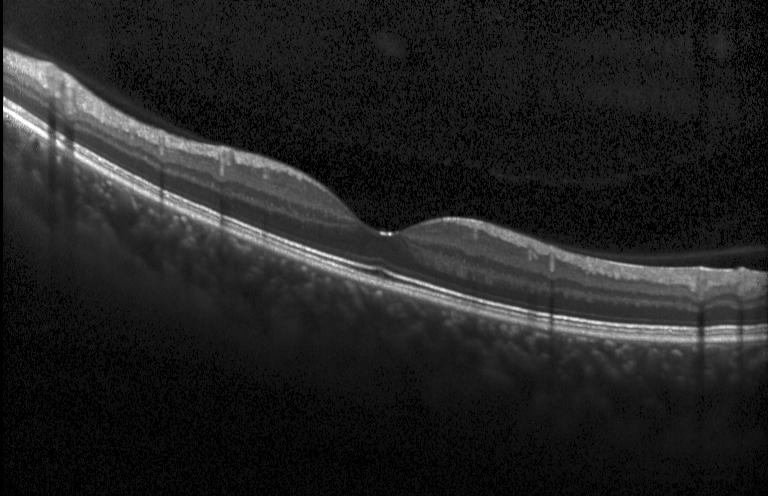

Optical coherence tomography B-scan · spectral-domain OCT · Heidelberg Spectralis · macular scan
Finding: no CNV, no DME, and no drusen.